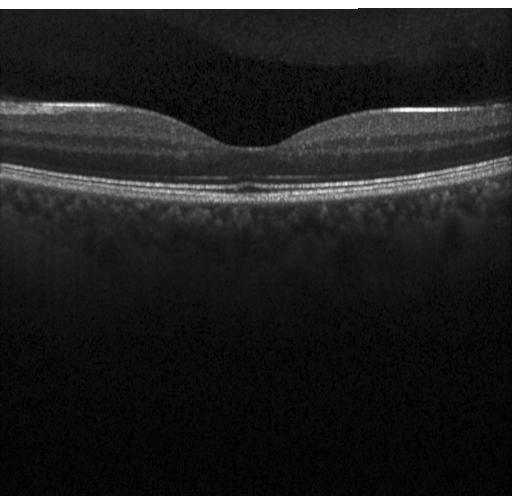

Retinal OCT B-scan. OCT finding: no evidence of choroidal neovascularization, diabetic macular edema, or drusen.